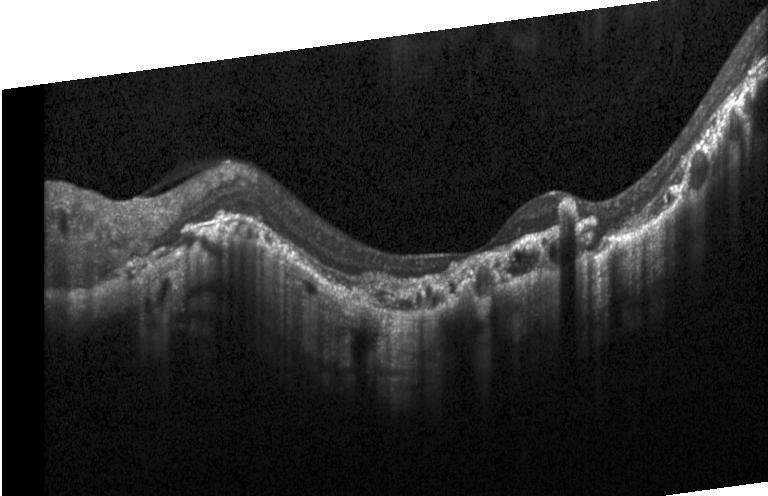 SD-OCT · Heidelberg Spectralis OCT system · retinal OCT B-scan · macular scan
CNV.